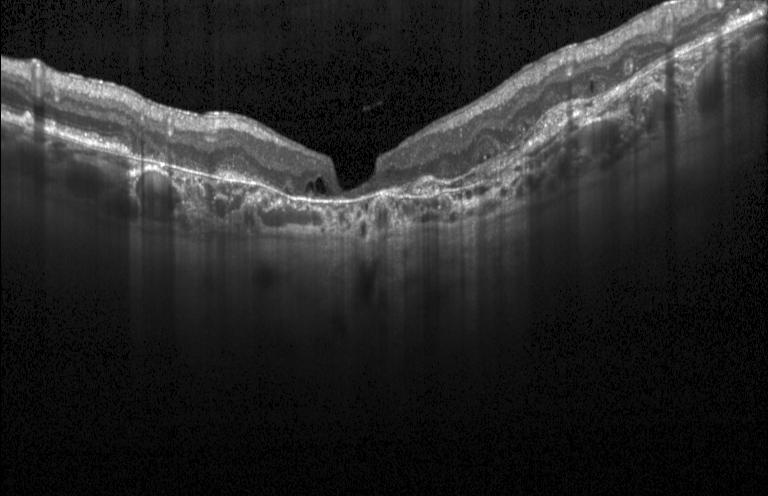
Dx: CNV.